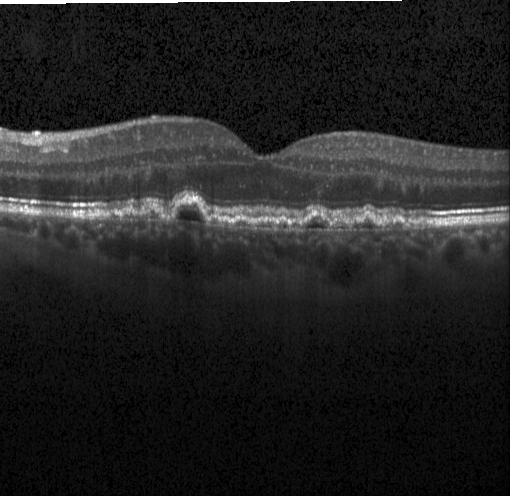

Optical coherence tomography B-scan, macular scan, acquired on a Heidelberg Spectralis. Finding: multiple drusen.